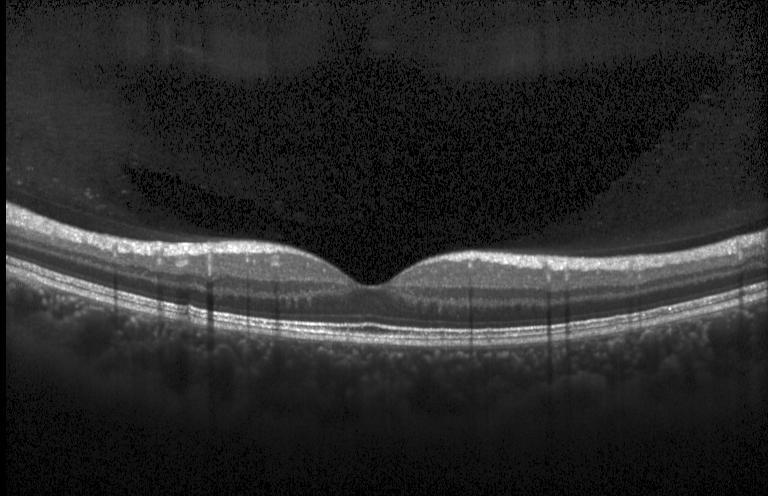

Heidelberg Spectralis; spectral-domain OCT; fovea-centered; retinal OCT B-scan. Impression: no evidence of choroidal neovascularization, diabetic macular edema, or drusen.